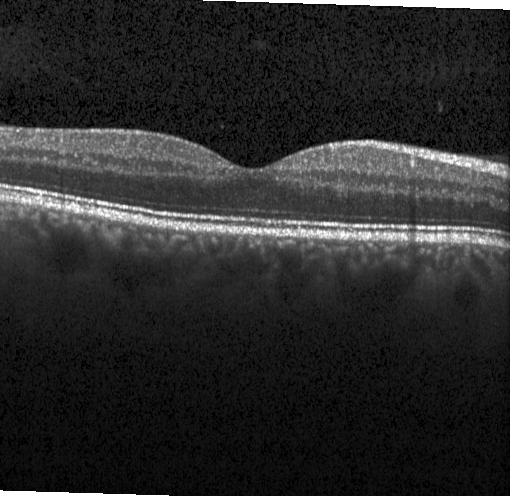 Macular OCT demonstrating neither choroidal neovascularization, diabetic macular edema, nor drusen.